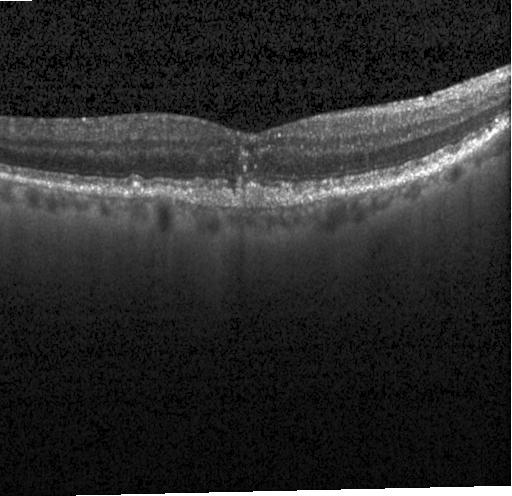 Retinal OCT cross-section. A choroidal neovascular membrane.